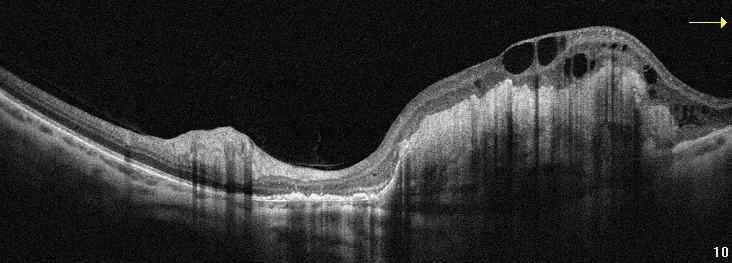

Age-related macular degeneration.